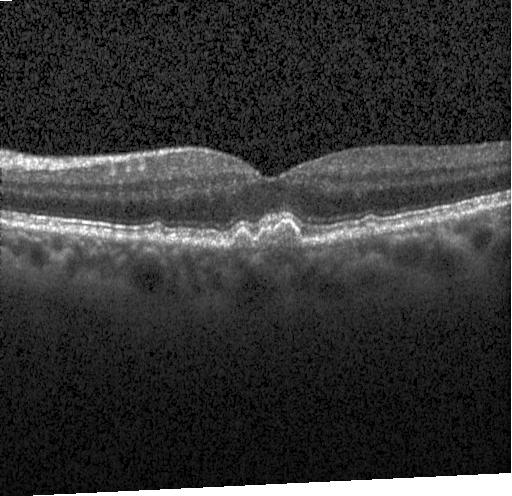

Optical coherence tomography B-scan
Multiple drusen.